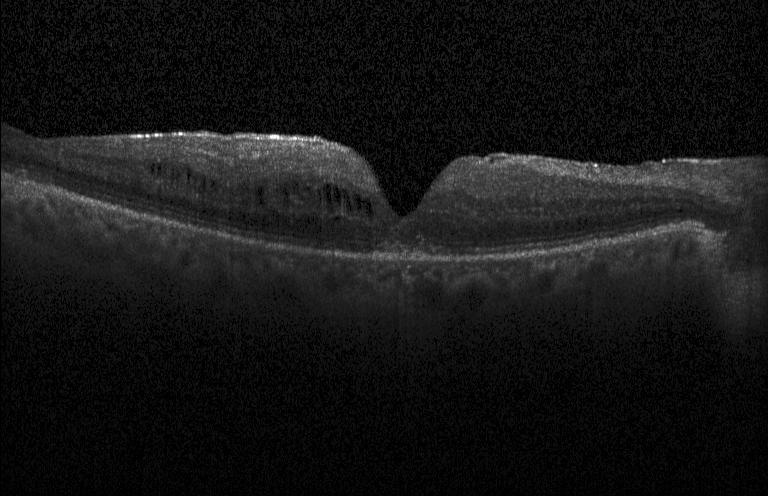
Optical coherence tomography scan, instrument: Heidelberg Spectralis — Macular OCT: DME.